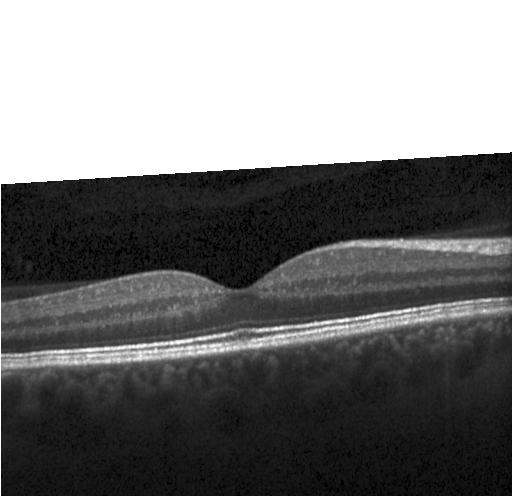
Heidelberg Spectralis OCT system; SD-OCT; OCT B-scan. Finding: no choroidal neovascularization, diabetic macular edema, or drusen.